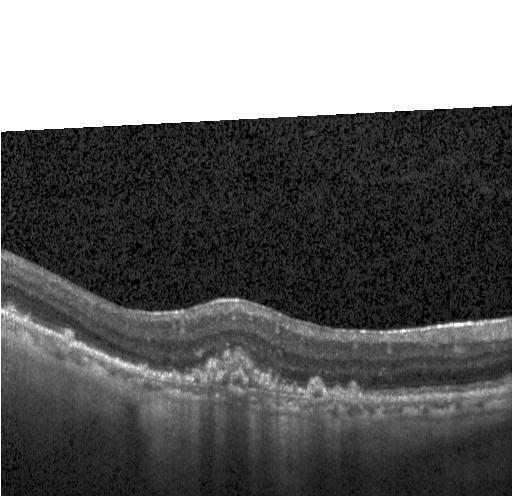
Assessment: choroidal neovascularization (CNV).